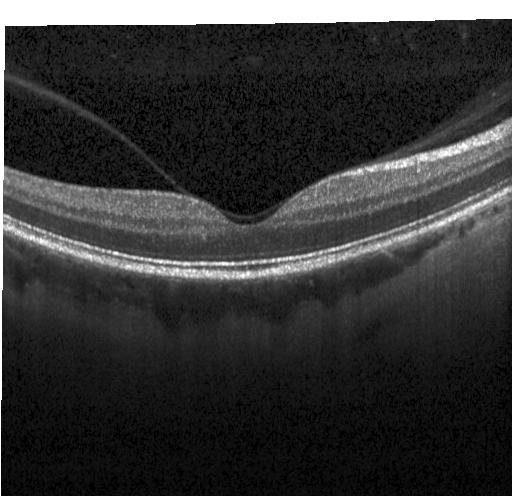
Finding: no choroidal neovascularization, diabetic macular edema, or drusen.